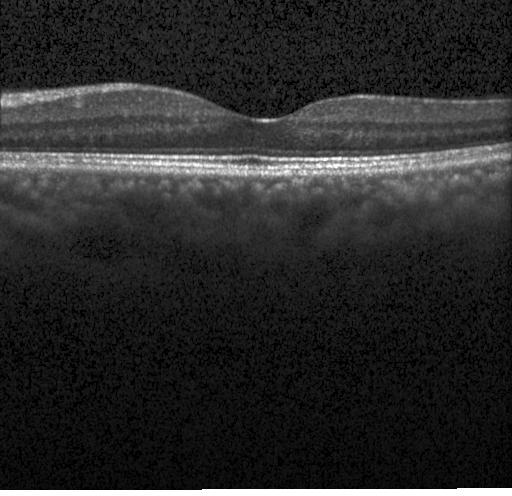

Optical coherence tomography scan; acquired on a Heidelberg Spectralis; spectral-domain OCT
Assessment: no evidence of choroidal neovascularization, diabetic macular edema, or drusen.